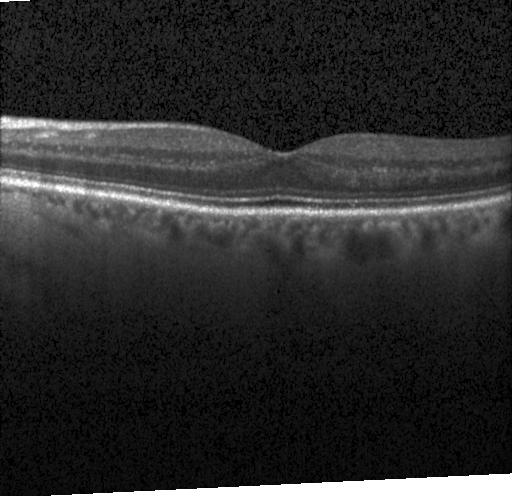

No evidence of choroidal neovascularization, diabetic macular edema, or drusen.